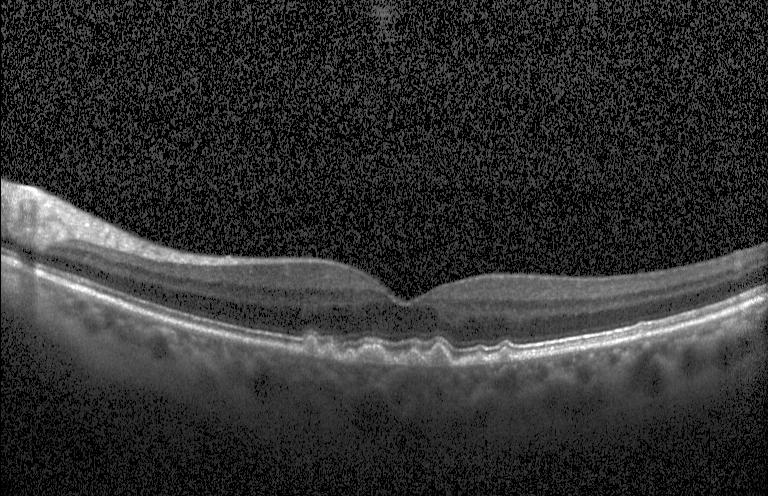

Macular OCT: drusen.